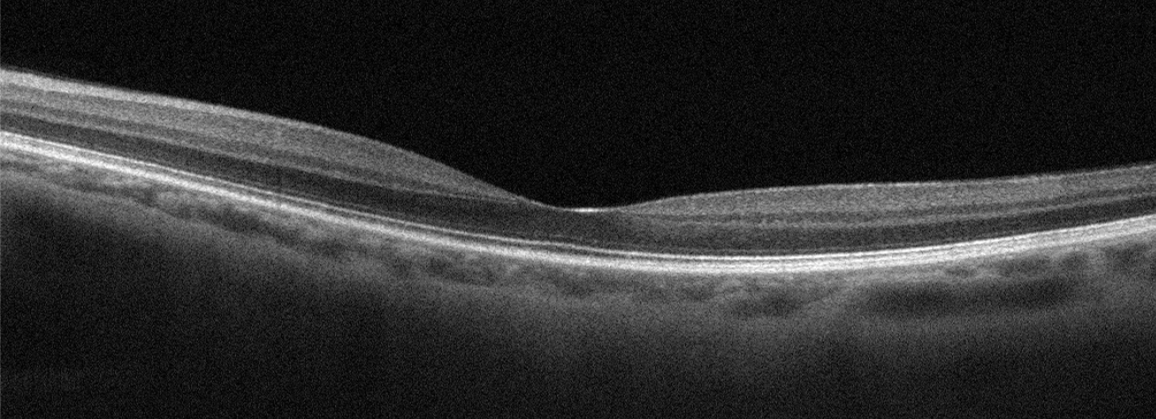
OCT scan showing no AMD, DME, ERM, RAO, RVO, or VID.